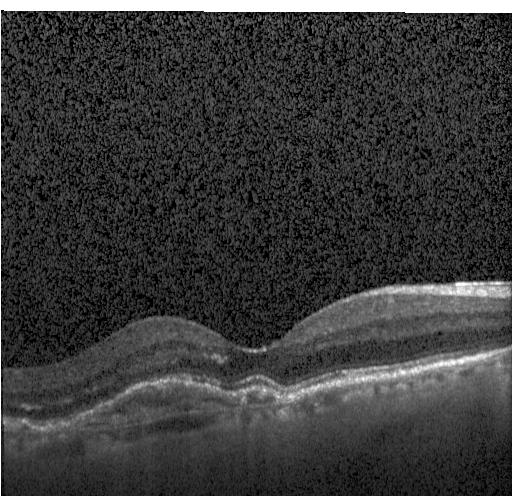 Spectral-domain OCT. Optical coherence tomography B-scan. Through the macula. Assessment: a choroidal neovascular membrane.